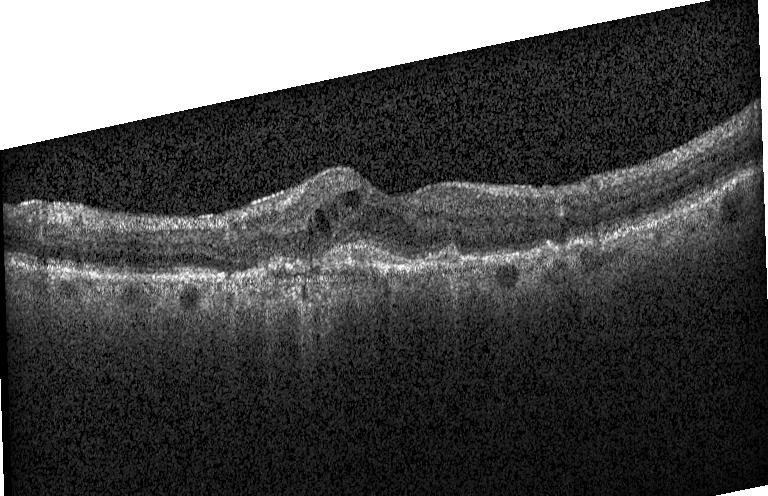
OCT B-scan showing a choroidal neovascular membrane.